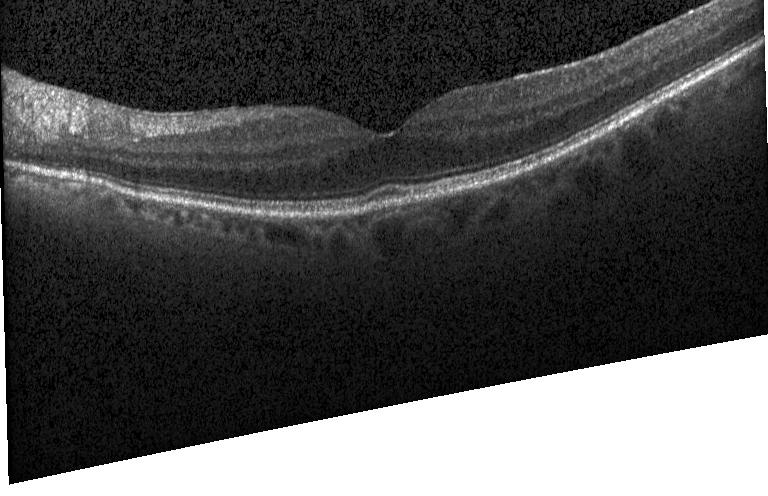

Centered on the fovea · Heidelberg Spectralis · optical coherence tomography scan. Impression: no evidence of choroidal neovascularization, diabetic macular edema, or drusen.